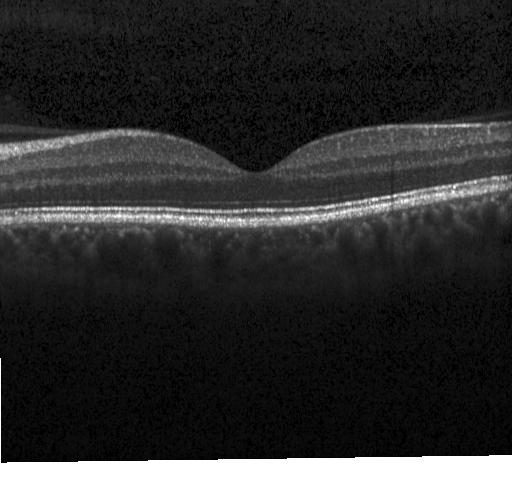
SD-OCT · OCT B-scan — Diagnosis: no choroidal neovascularization, diabetic macular edema, or drusen.